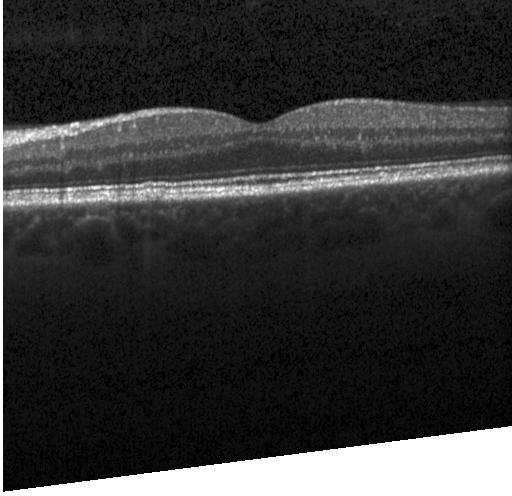 Dx: neither CNV, DME, nor drusen.